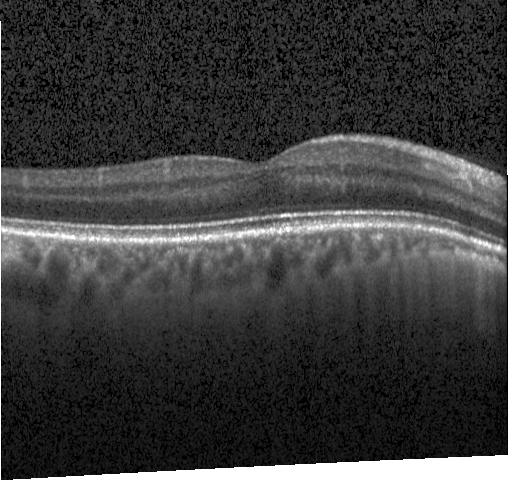

Optical coherence tomography B-scan.
The scan shows no evidence of CNV, DME, or drusen.